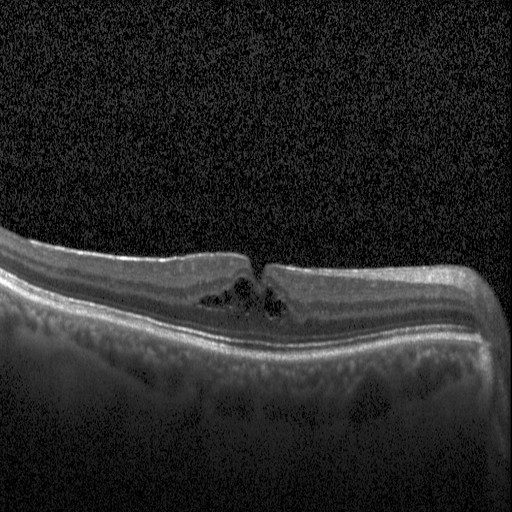 SD-OCT. OCT B-scan
Dx: diabetic macular edema.